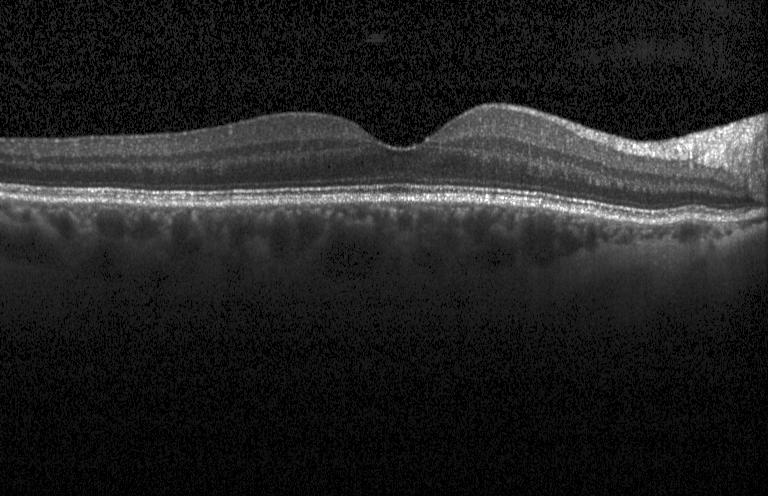

Macular OCT demonstrating no choroidal neovascularization, no diabetic macular edema, and no drusen.